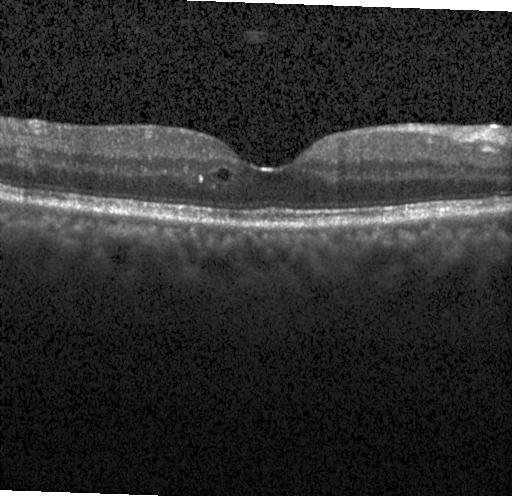
This B-scan demonstrates DME.